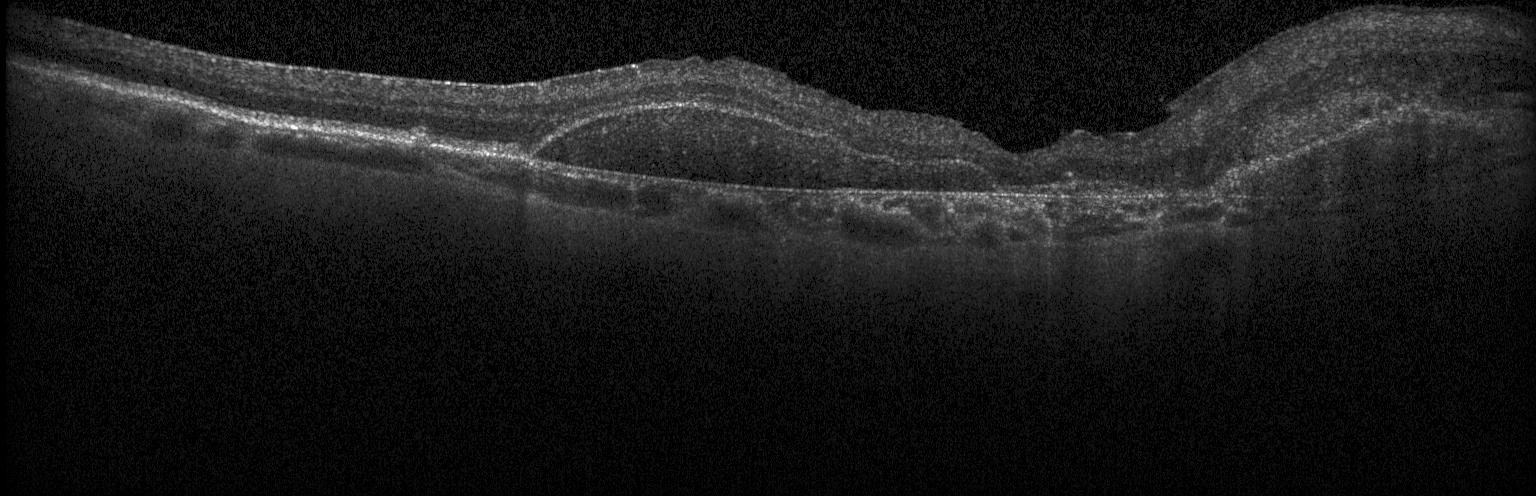
OCT B-scan.
Assessment: choroidal neovascularization.